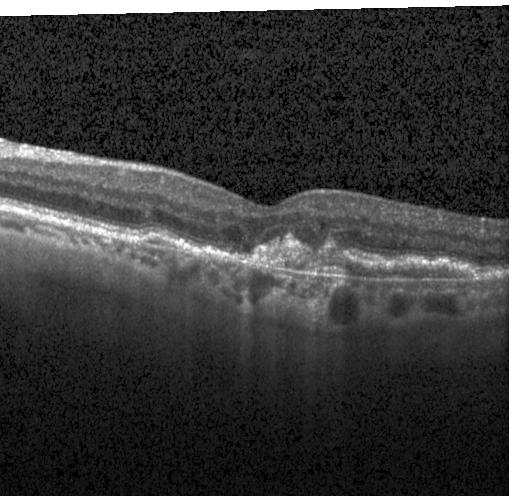
Optical coherence tomography B-scan · instrument: Heidelberg Spectralis — This B-scan demonstrates CNV.